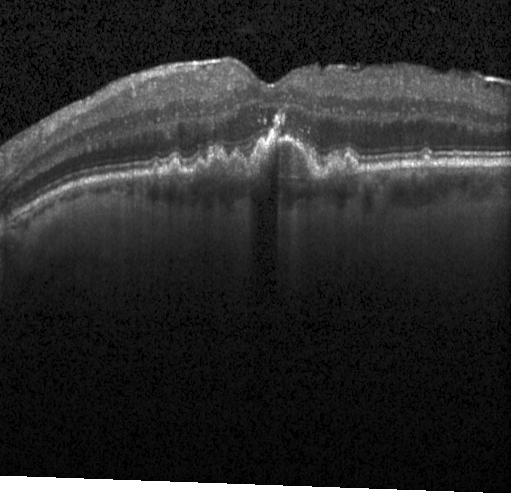

OCT line scan, acquired on a Heidelberg Spectralis. Impression: sub-RPE drusenoid deposits.